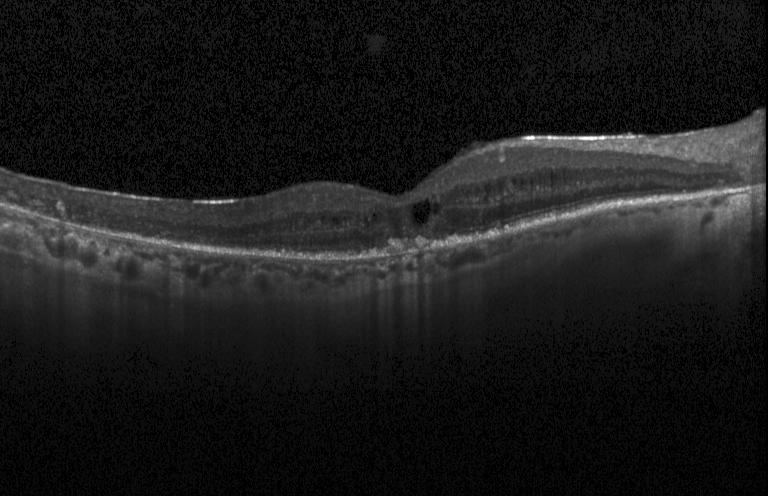
This B-scan demonstrates a choroidal neovascular membrane.